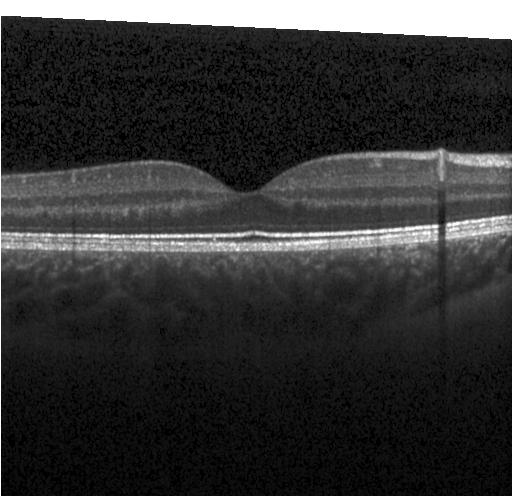

OCT B-scan; horizontal scan through the fovea; Heidelberg Spectralis
Impression: no choroidal neovascularization, no diabetic macular edema, and no drusen.